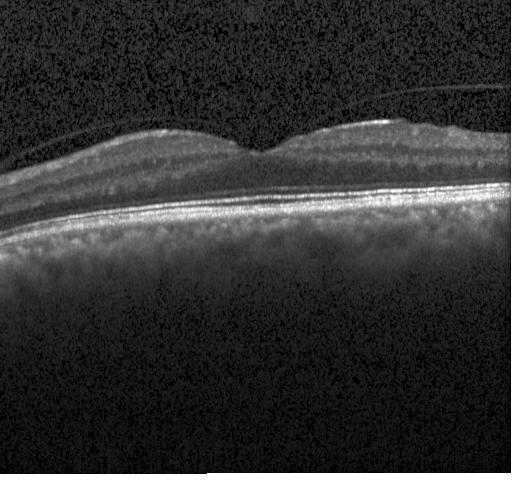 Retinal OCT cross-section; fovea-centered; Heidelberg Spectralis OCT system; SD-OCT — The scan shows neither CNV, DME, nor drusen.